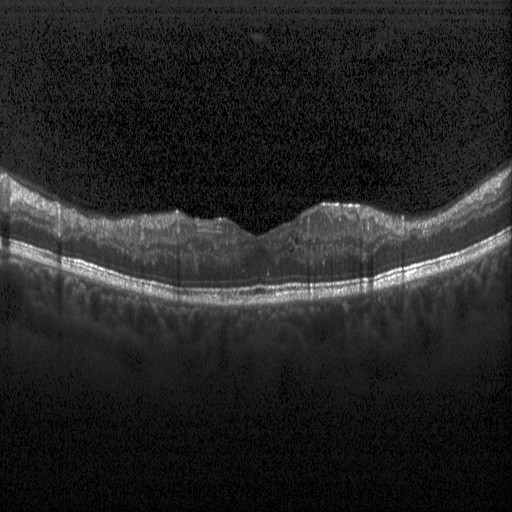
Assessment: diabetic macular edema (DME).